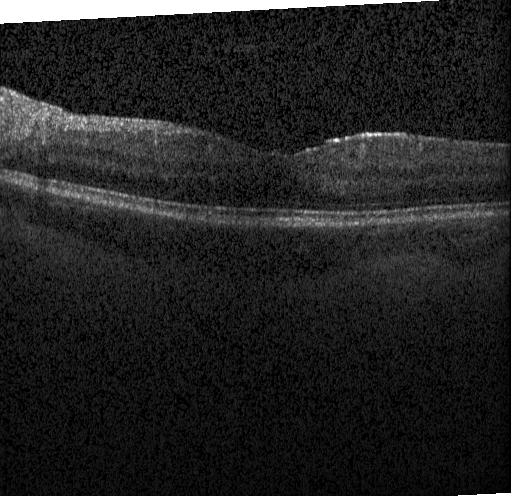 Heidelberg Spectralis · OCT line scan · spectral-domain OCT
Macular OCT: neither choroidal neovascularization, diabetic macular edema, nor drusen.